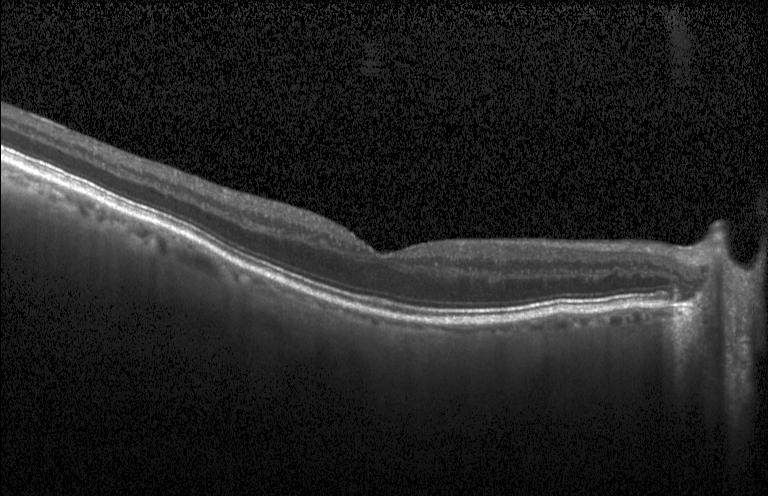
Finding: neither CNV, DME, nor drusen.